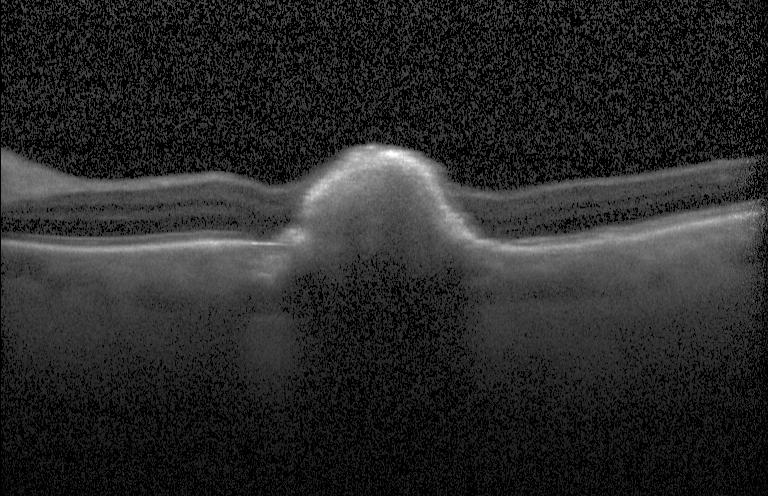

Diagnosis: CNV.